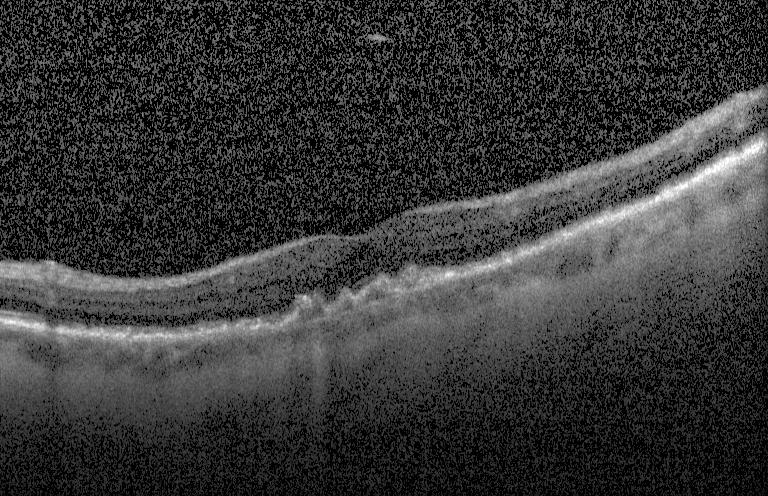
Retinal OCT B-scan; through the macula — Impression: a choroidal neovascular membrane.